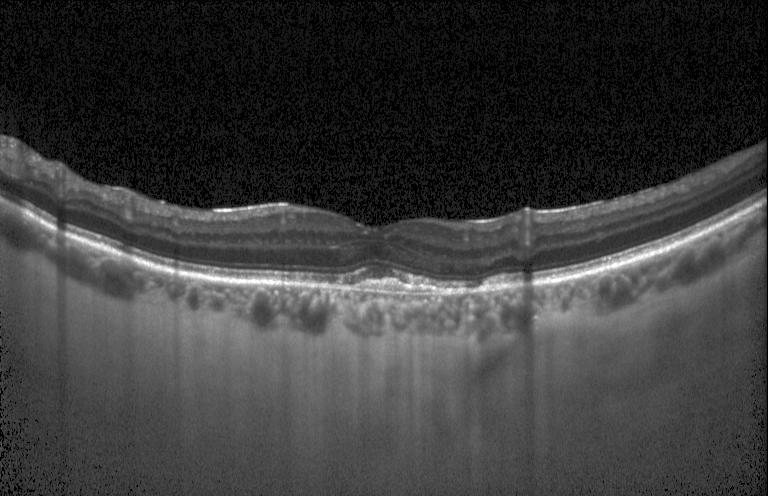
Impression: CNV.